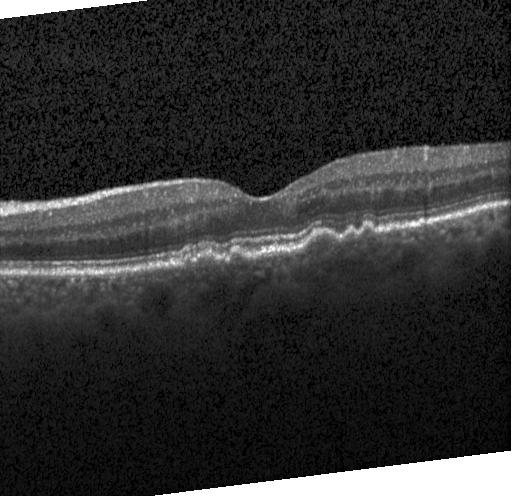
Multiple drusen.